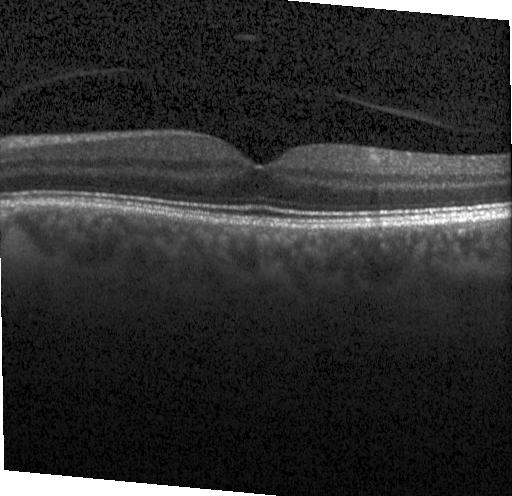
Retinal OCT cross-section. Centered on the fovea. Heidelberg Spectralis
Dx: no CNV, DME, or drusen.